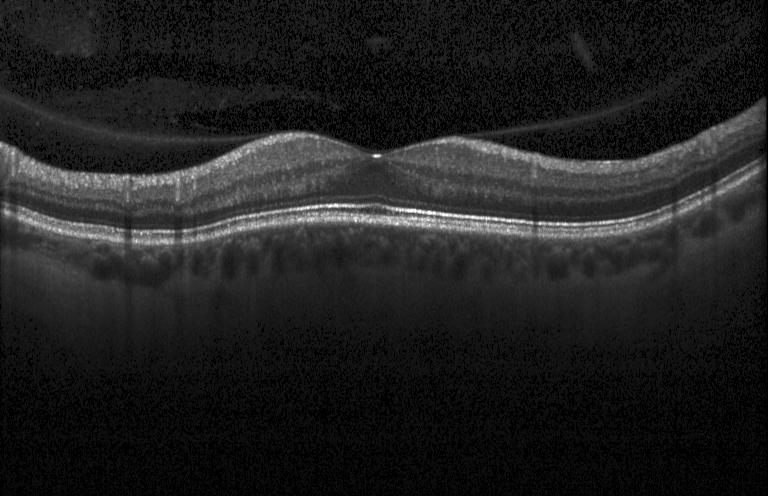

SD-OCT · retinal OCT cross-section.
Macular OCT: no CNV, no DME, and no drusen.